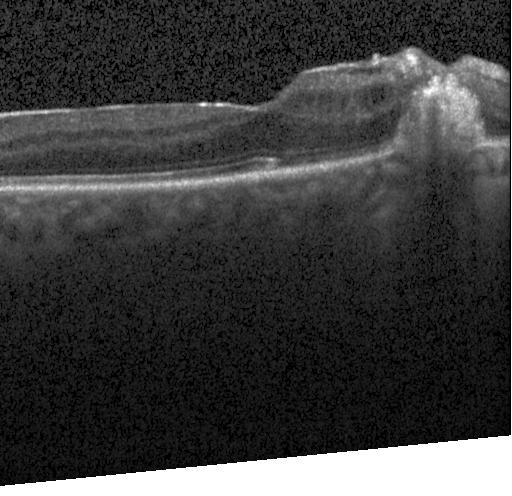

Heidelberg Spectralis OCT system, OCT line scan, spectral-domain OCT
Dx: a choroidal neovascular membrane.